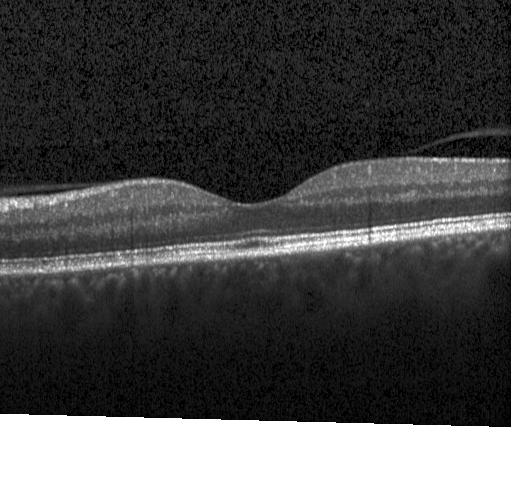 Finding: no evidence of CNV, DME, or drusen.